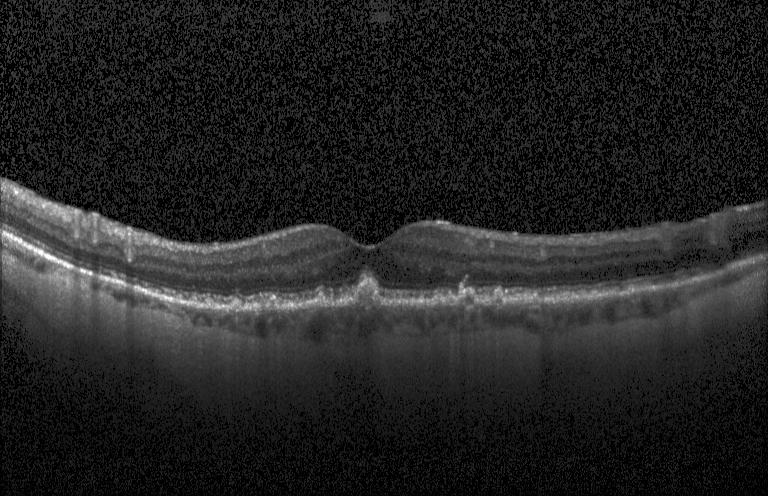 OCT B-scan — Impression: drusen.